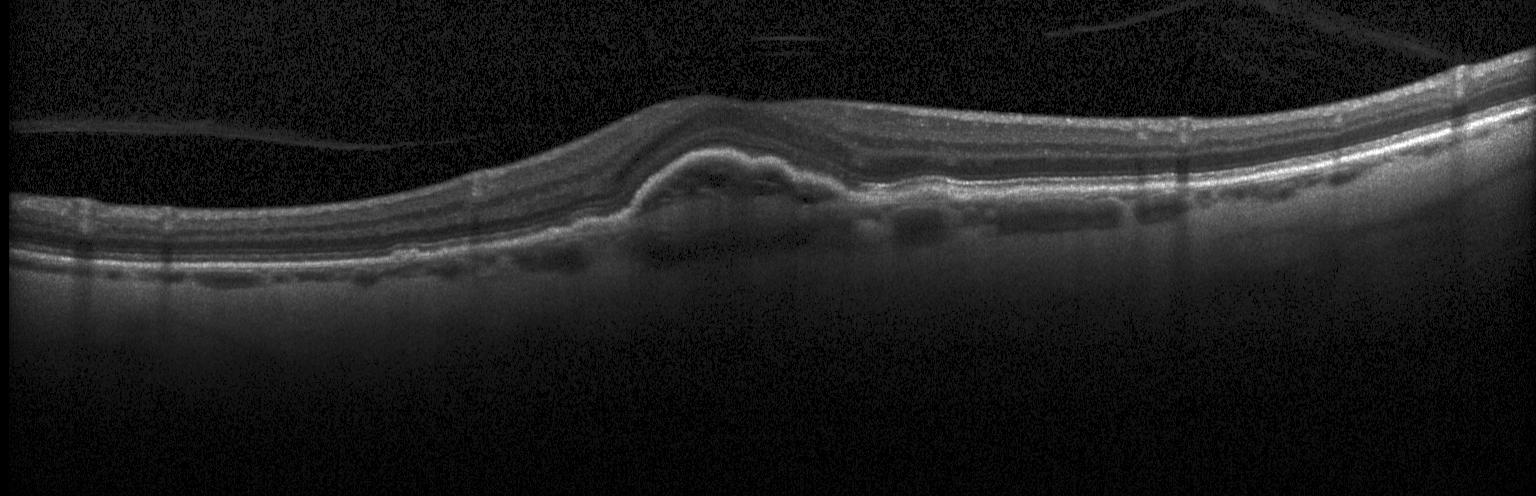

Spectral-domain optical coherence tomography, optical coherence tomography scan, Heidelberg Spectralis OCT system.
Impression: a choroidal neovascular membrane.